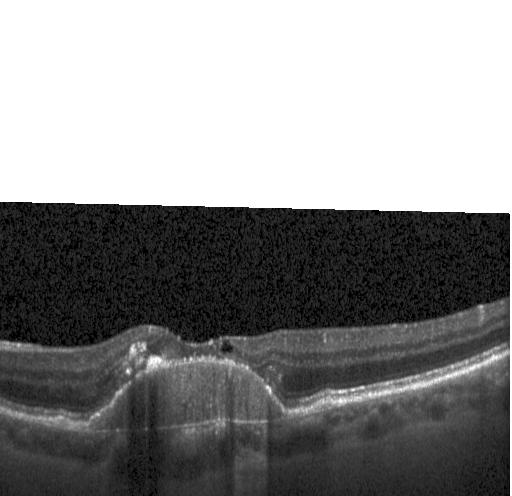
Spectral-domain OCT, OCT line scan, instrument: Heidelberg Spectralis, centered on the fovea — Dx: CNV.